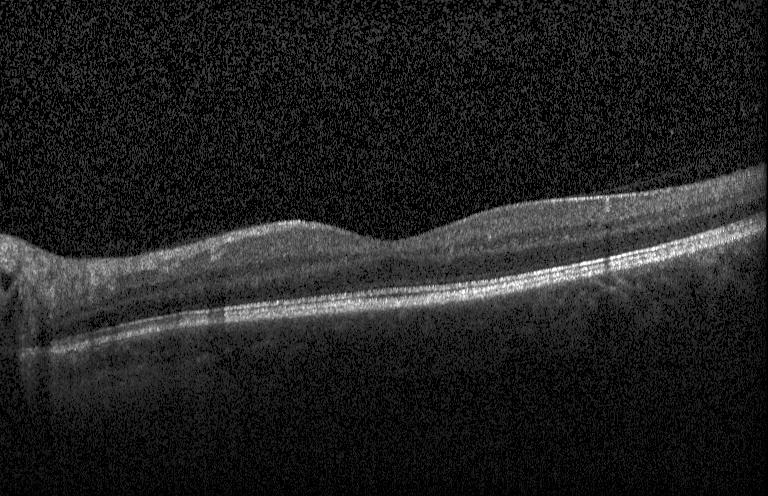
Diagnosis: no CNV, no DME, and no drusen.